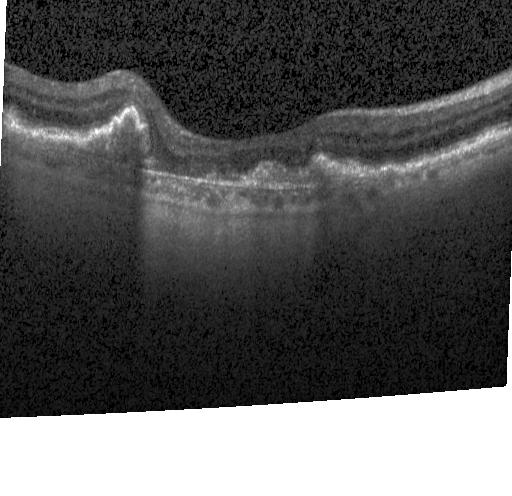 Macular OCT: CNV.